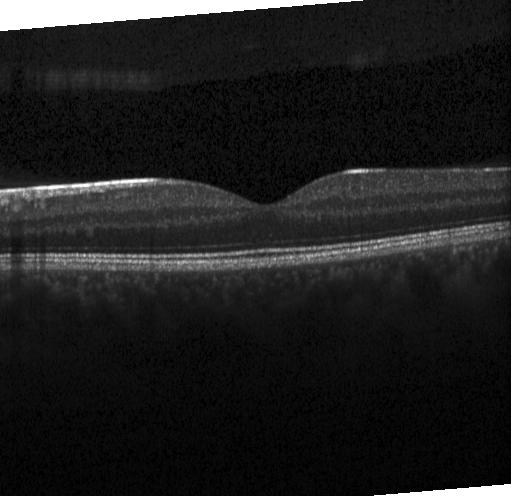 Fovea-centered, acquired on a Heidelberg Spectralis, retinal OCT cross-section, SD-OCT.
Assessment: neither choroidal neovascularization, diabetic macular edema, nor drusen.